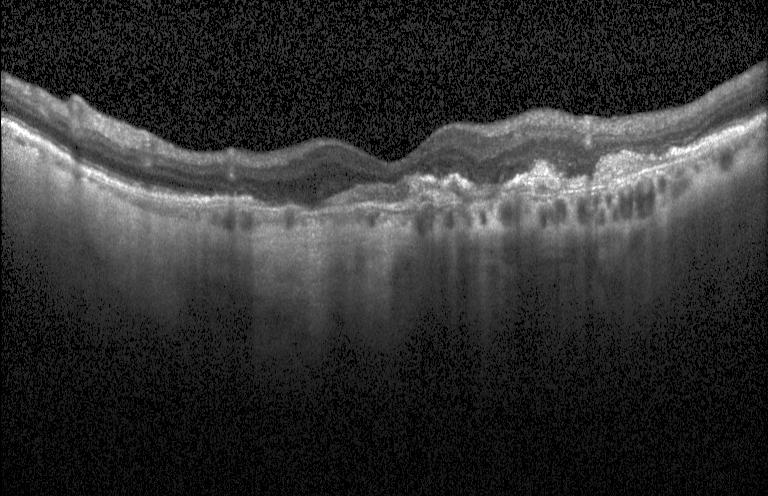

Dx: choroidal neovascularization (CNV).